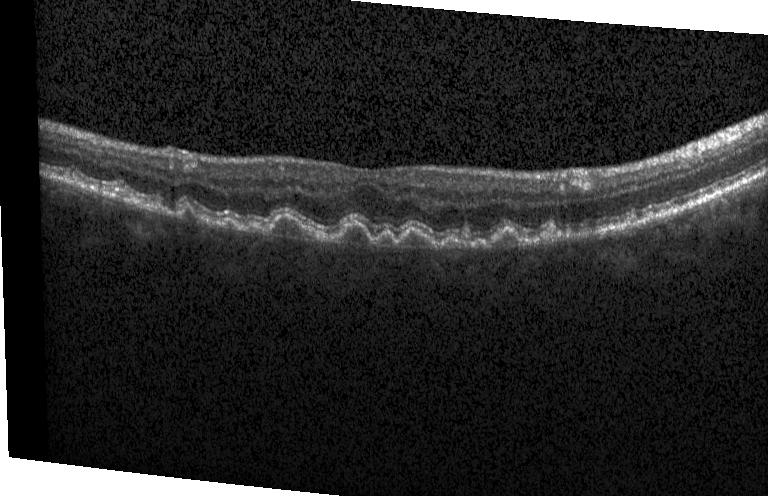 OCT B-scan. Through the macula. Instrument: Heidelberg Spectralis. Spectral-domain OCT — This B-scan demonstrates drusen.